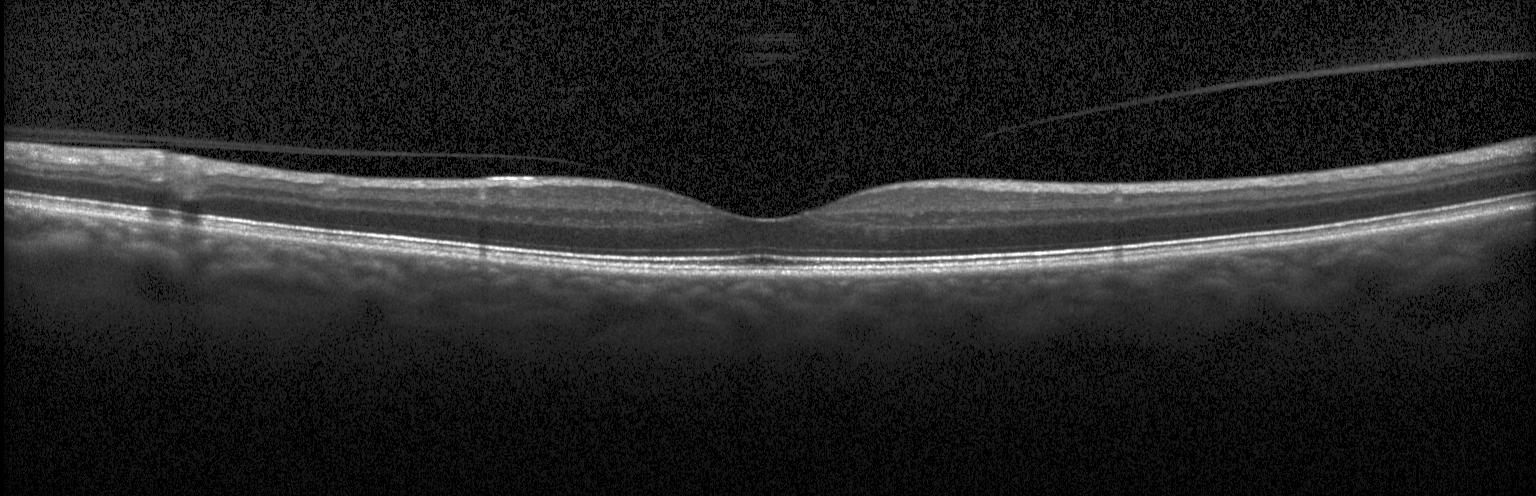
Retinal OCT cross-section. Impression: no evidence of CNV, DME, or drusen.